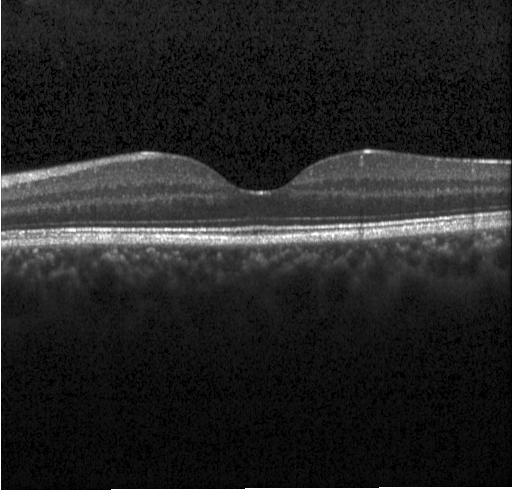 Retinal OCT B-scan
Impression: no CNV, no DME, and no drusen.